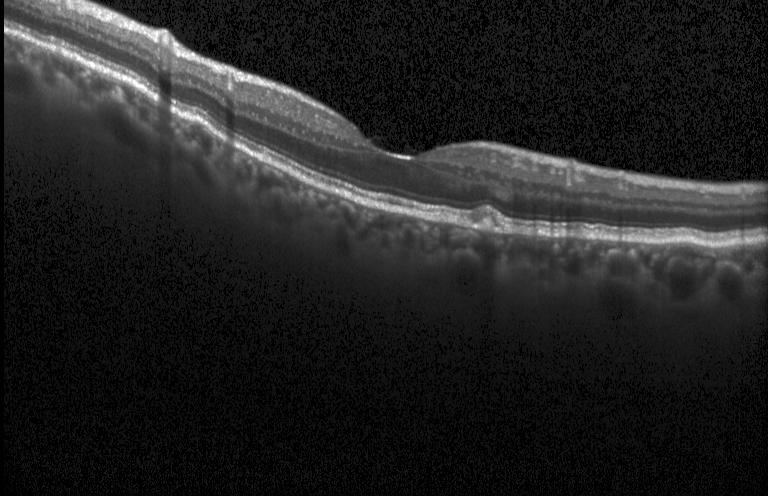

Impression: drusen.